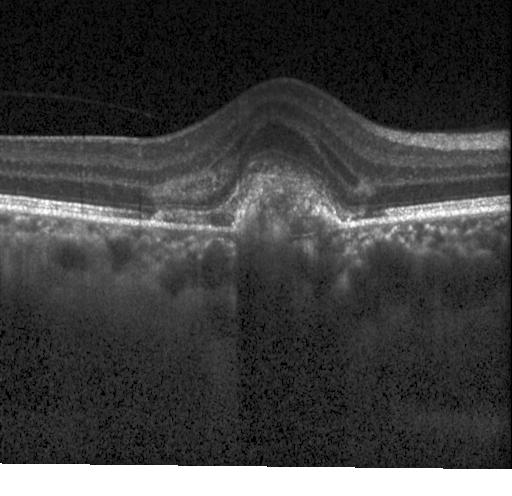 OCT line scan.
Diagnosis: a choroidal neovascular membrane.